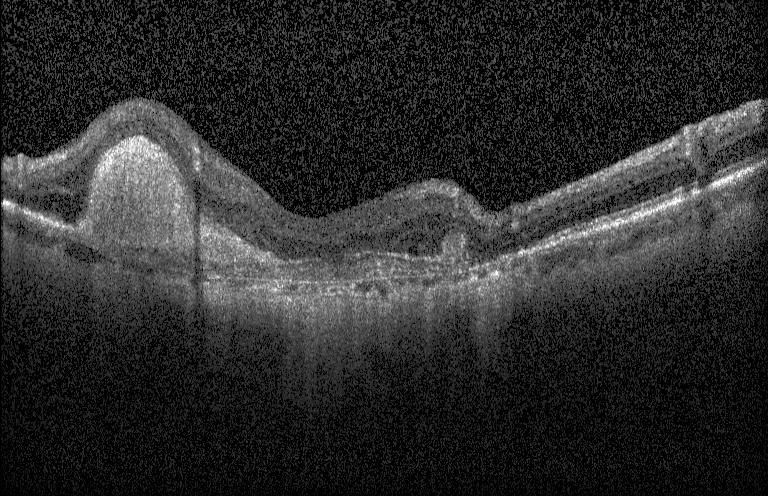
SD-OCT, optical coherence tomography scan
The scan shows choroidal neovascularization.